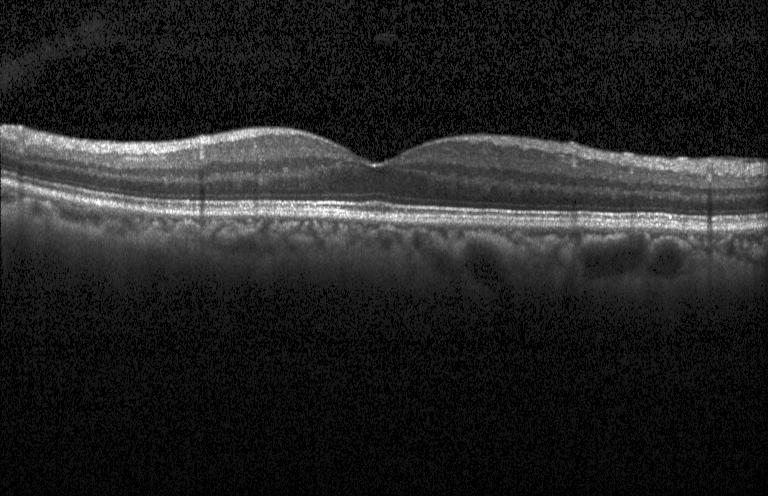

OCT B-scan
Assessment: neither CNV, DME, nor drusen.